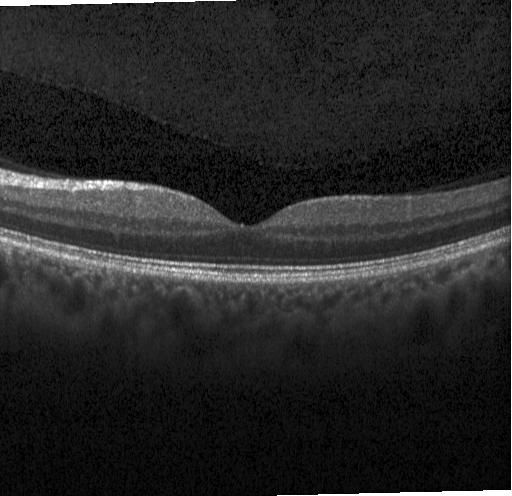 Dx: no choroidal neovascularization, diabetic macular edema, or drusen.